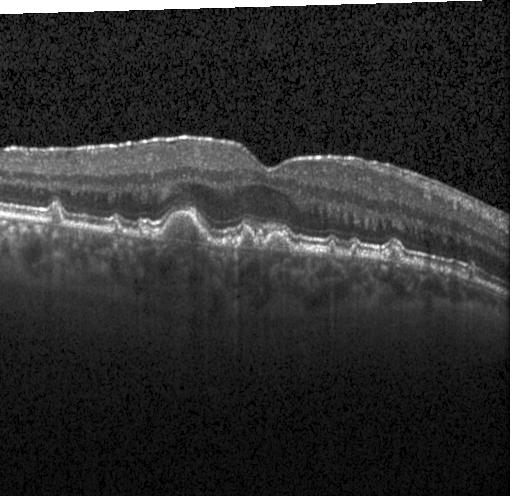
Retinal OCT cross-section — The scan shows multiple drusen.